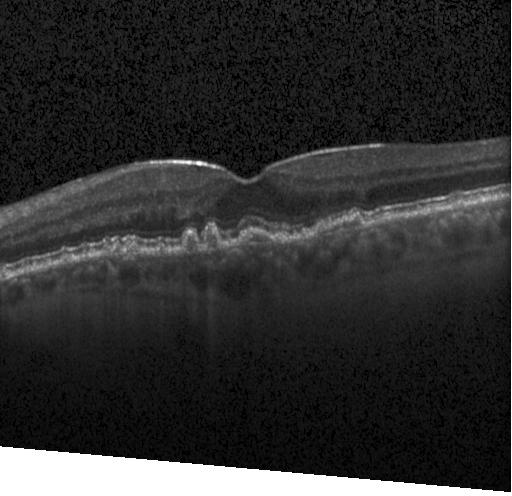

OCT line scan; horizontal scan through the fovea — The scan shows sub-RPE drusenoid deposits.